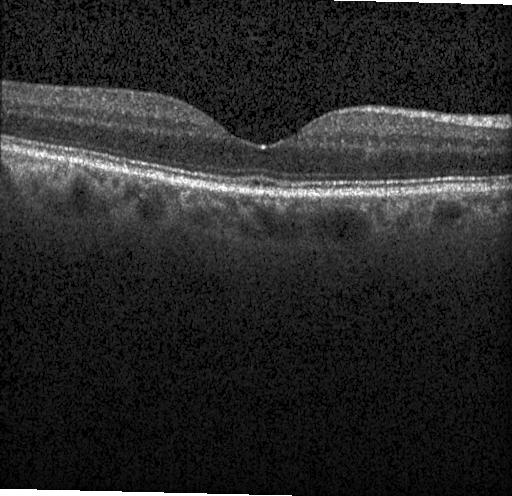
This B-scan demonstrates no evidence of choroidal neovascularization, diabetic macular edema, or drusen.